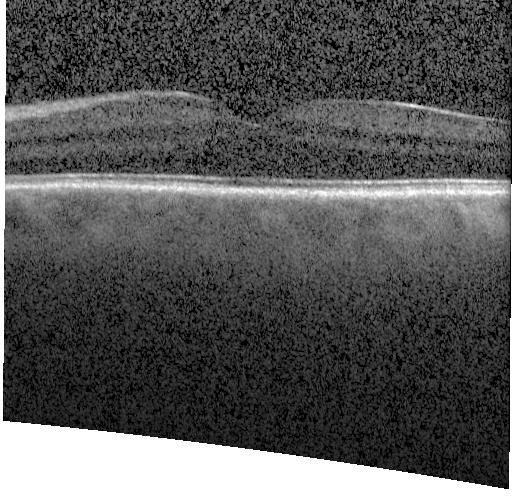
Diagnosis: no evidence of CNV, DME, or drusen.